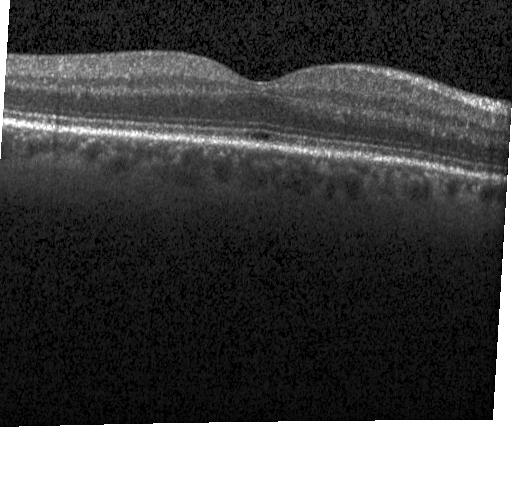

Centered on the fovea, retinal OCT cross-section, Heidelberg Spectralis OCT system. Diagnosis: no CNV, no DME, and no drusen.